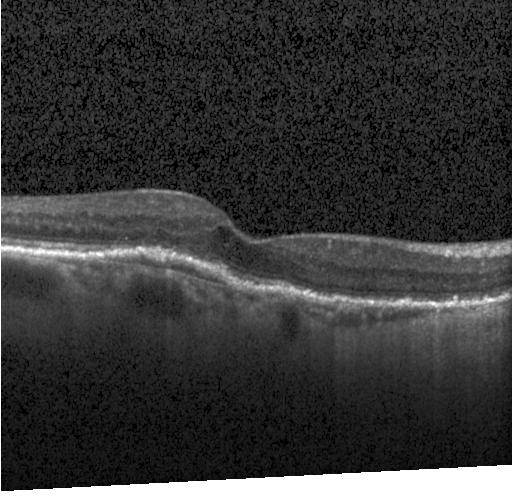
OCT B-scan. The scan shows choroidal neovascularization (CNV).